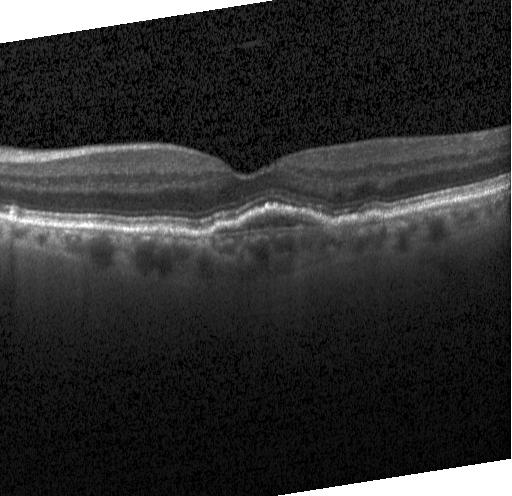 Spectral-domain OCT · OCT line scan · horizontal scan through the fovea
OCT finding: choroidal neovascularization (CNV).